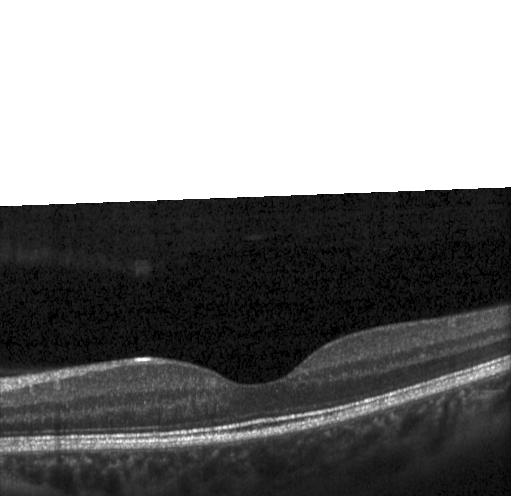 Optical coherence tomography B-scan · centered on the fovea · spectral-domain optical coherence tomography. Impression: no CNV, no DME, and no drusen.